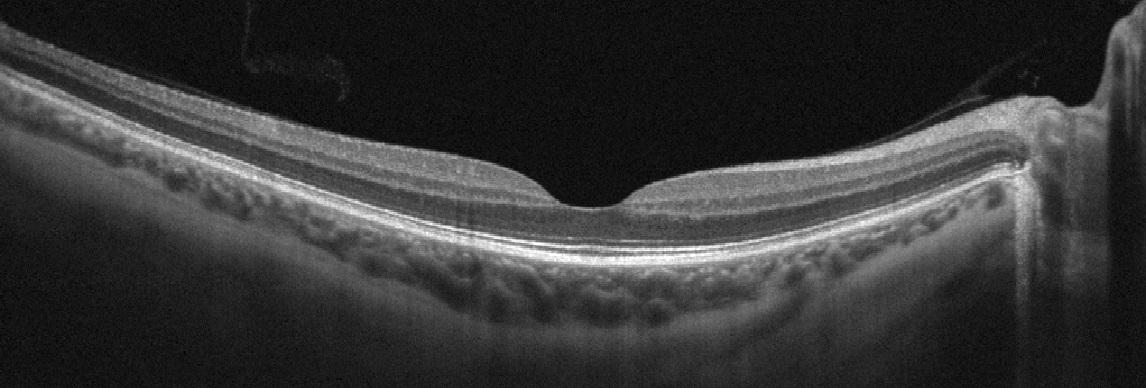

Fovea-centered, OCT line scan. Impression: no evidence of AMD, DME, ERM, RAO, RVO, or VID.